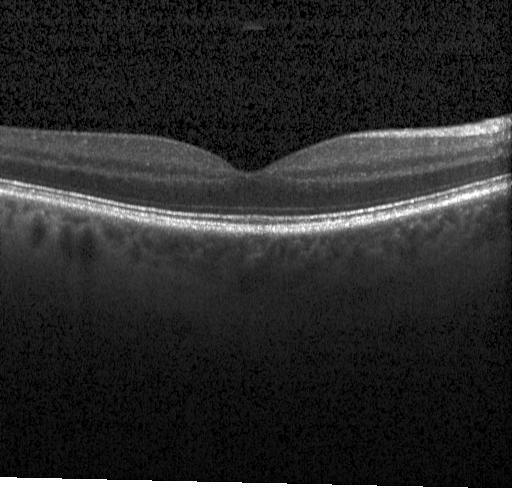
Retinal OCT cross-section showing neither choroidal neovascularization, diabetic macular edema, nor drusen.